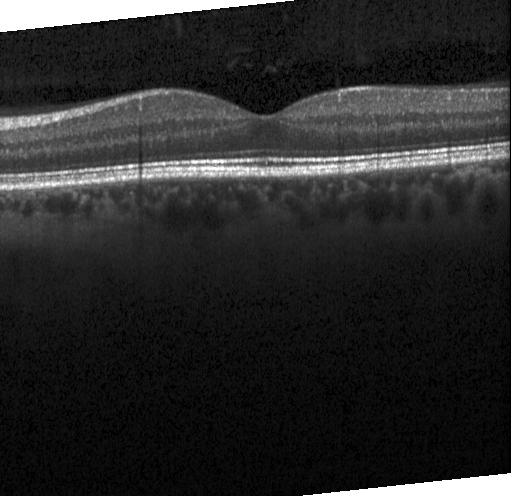
No evidence of CNV, DME, or drusen.